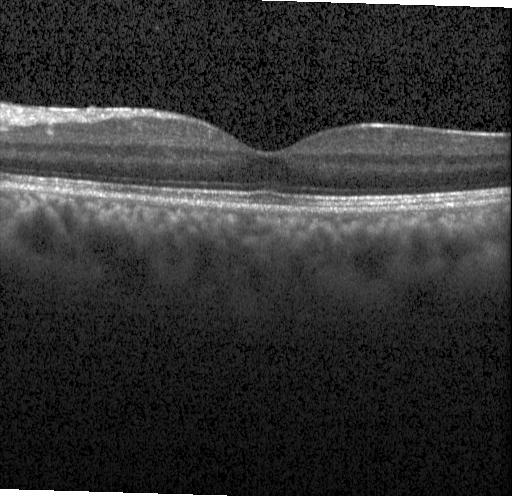

This B-scan demonstrates no choroidal neovascularization, diabetic macular edema, or drusen.